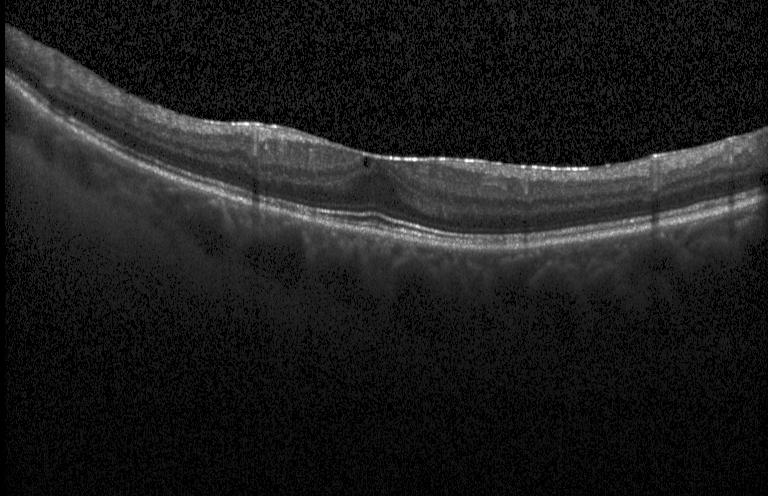
Horizontal scan through the fovea; instrument: Heidelberg Spectralis; retinal OCT cross-section; spectral-domain optical coherence tomography. Assessment: diabetic macular edema (DME).